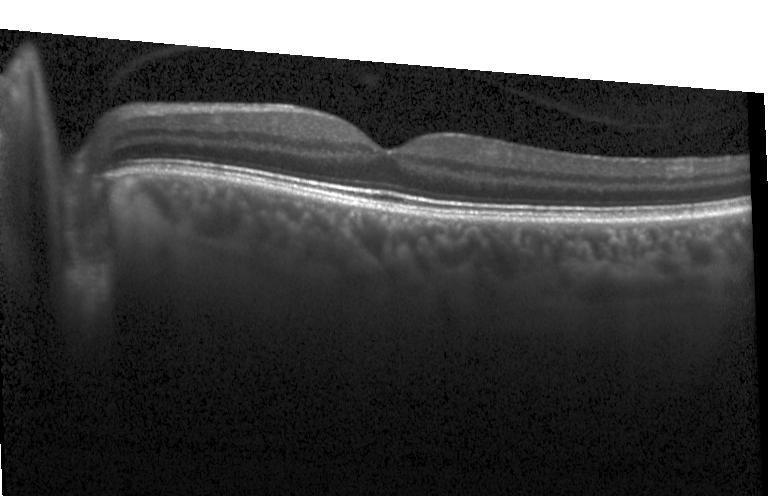
Macular OCT demonstrating no evidence of choroidal neovascularization, diabetic macular edema, or drusen.